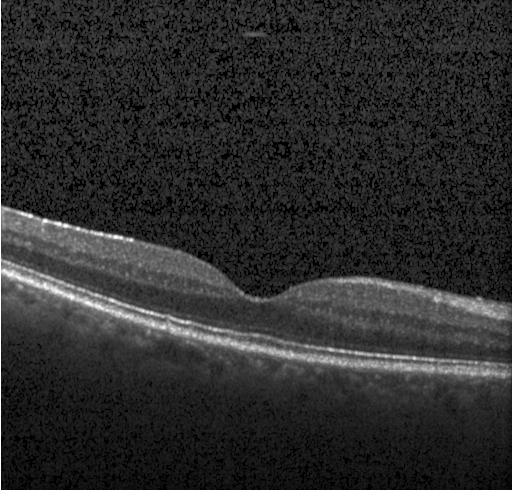 OCT B-scan.
Neither choroidal neovascularization, diabetic macular edema, nor drusen.